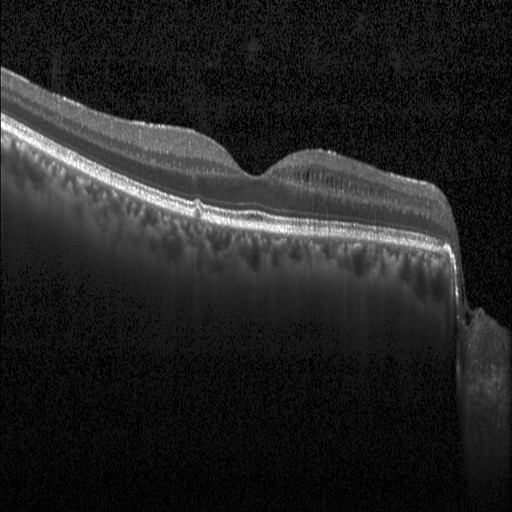

Spectral-domain optical coherence tomography · retinal OCT cross-section — Assessment: diabetic macular edema (DME).